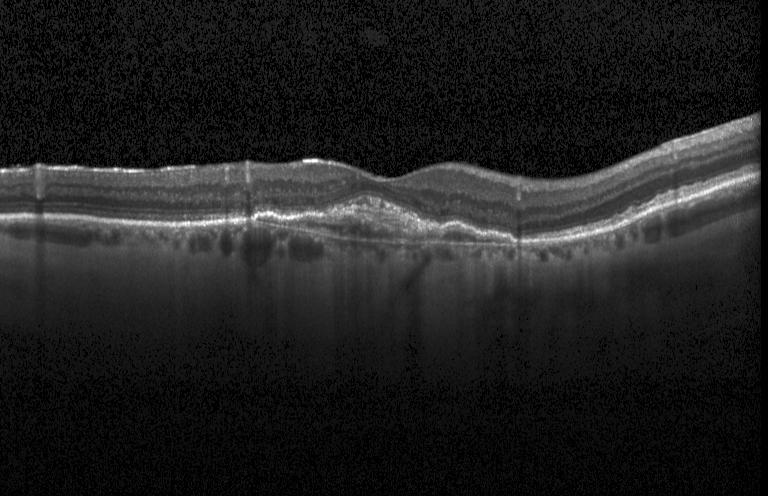
Through the macula; instrument: Heidelberg Spectralis; spectral-domain OCT; retinal OCT B-scan. Assessment: a choroidal neovascular membrane.